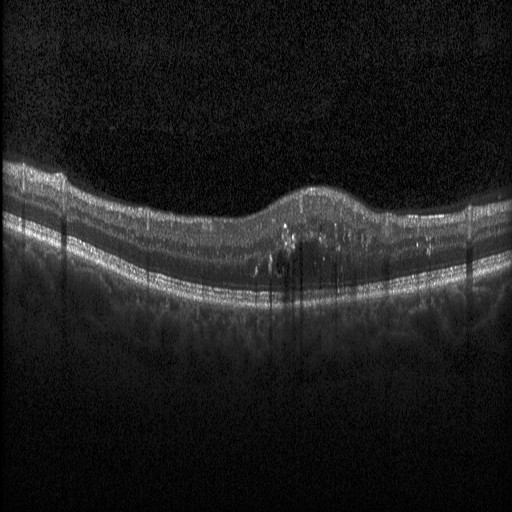
Macular OCT demonstrating diabetic macular edema (DME).